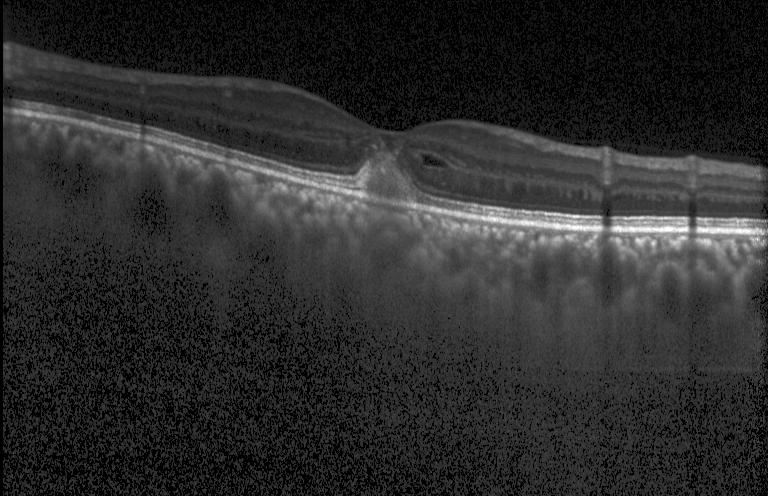 Retinal OCT cross-section showing choroidal neovascularization.